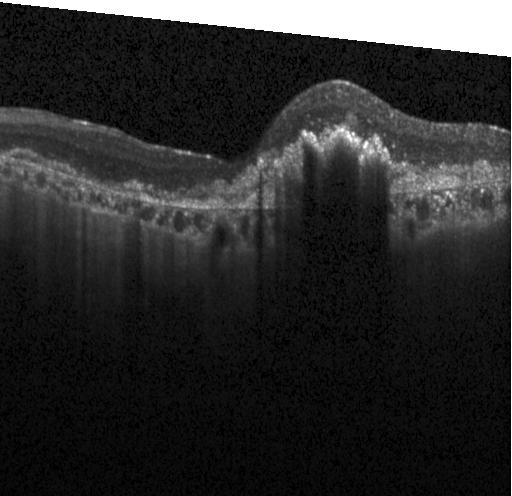
OCT B-scan showing a choroidal neovascular membrane.